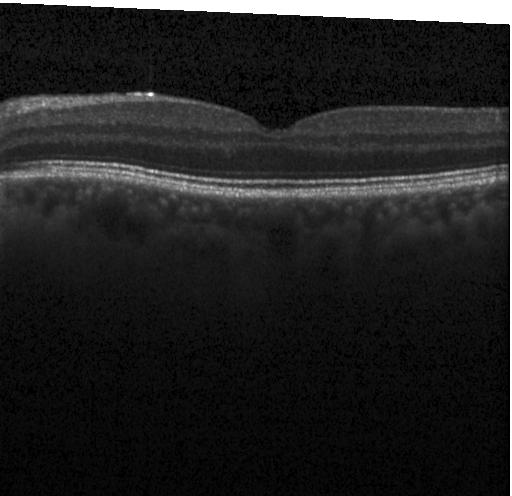
Macular scan · optical coherence tomography B-scan · Heidelberg Spectralis OCT system · spectral-domain OCT. Dx: no choroidal neovascularization, no diabetic macular edema, and no drusen.